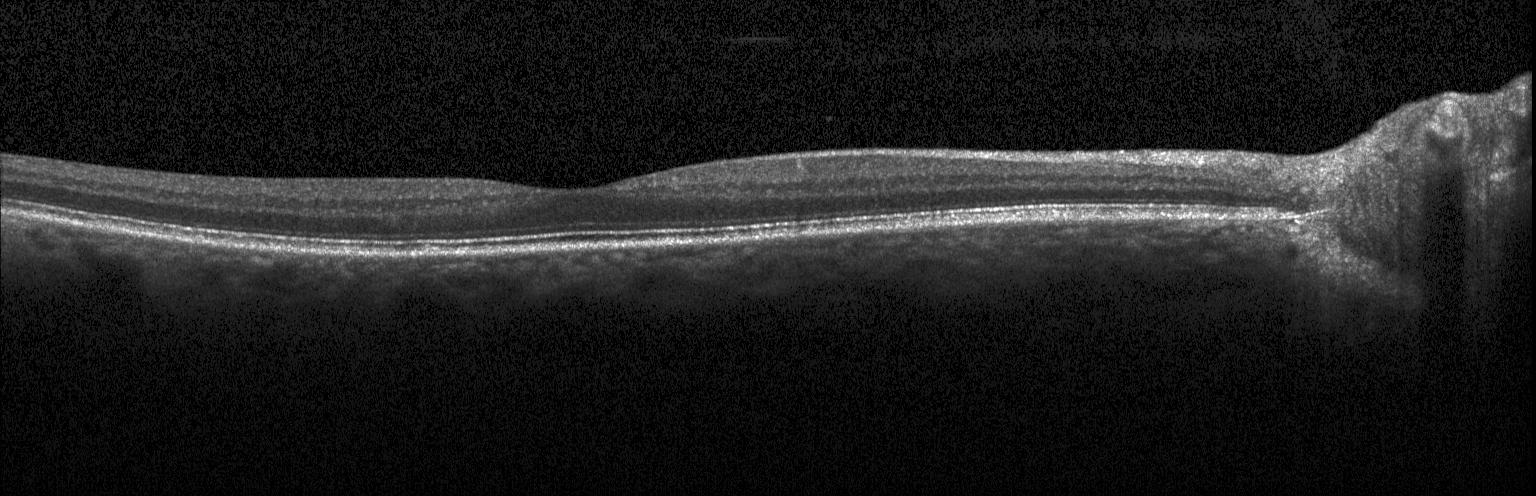 Centered on the fovea, OCT B-scan, spectral-domain optical coherence tomography, Heidelberg Spectralis OCT system — Diagnosis: no evidence of choroidal neovascularization, diabetic macular edema, or drusen.